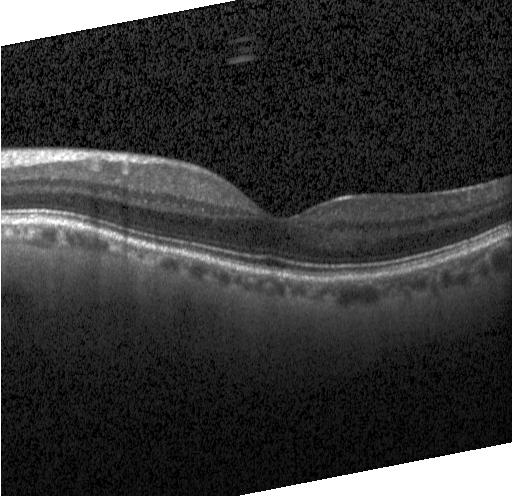

Horizontal scan through the fovea; retinal OCT B-scan; acquired on a Heidelberg Spectralis
Finding: no choroidal neovascularization, no diabetic macular edema, and no drusen.